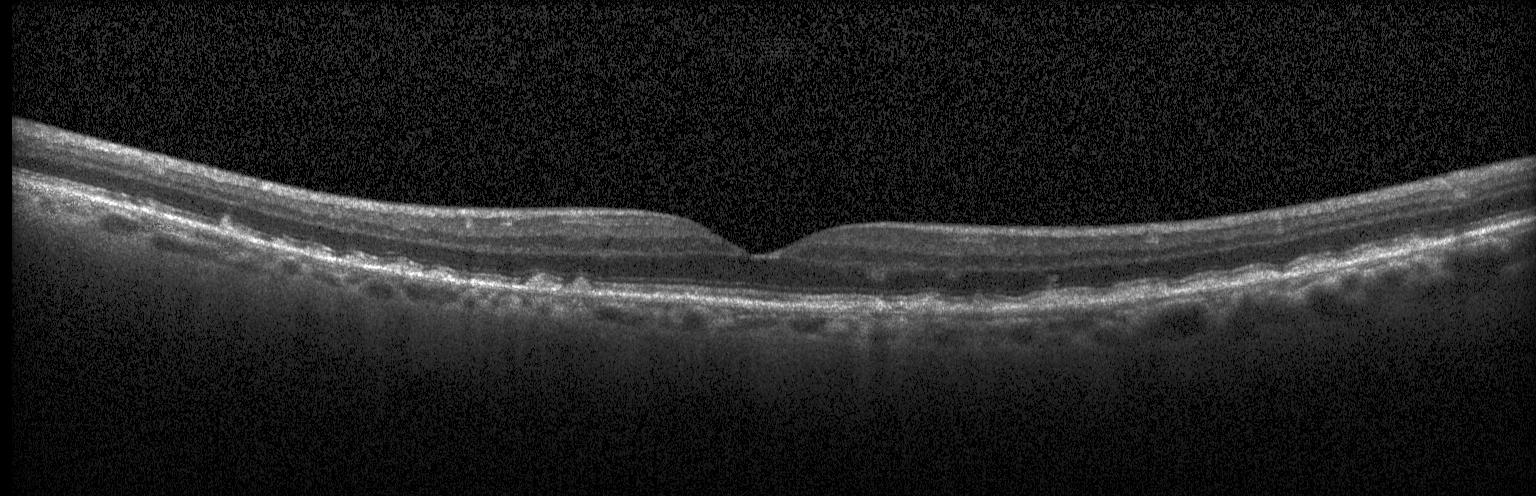
Sub-RPE drusenoid deposits.